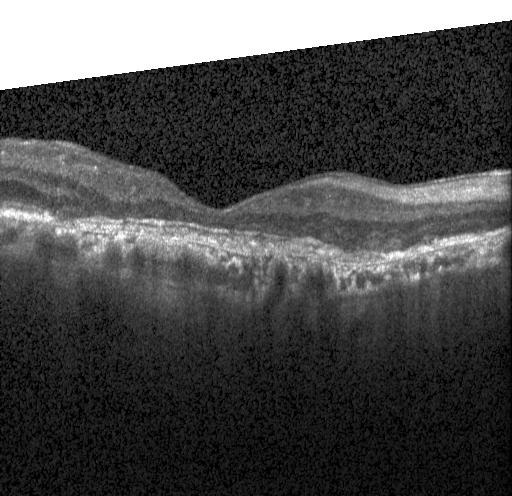 OCT B-scan showing choroidal neovascularization.